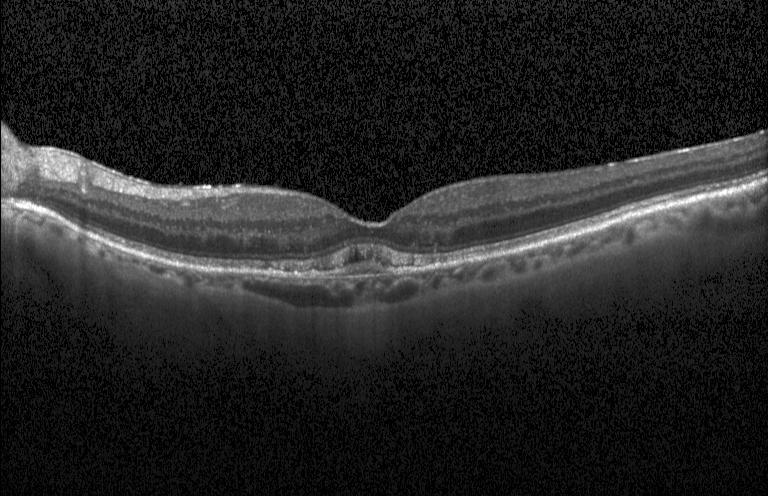
OCT B-scan; fovea-centered; spectral-domain optical coherence tomography; acquired on a Heidelberg Spectralis — Finding: a choroidal neovascular membrane.